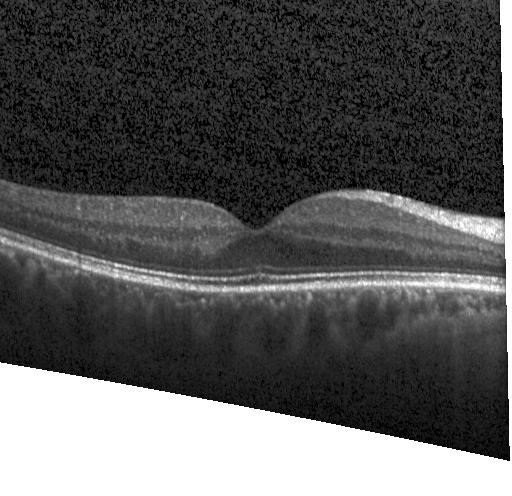
Diagnosis: no evidence of CNV, DME, or drusen.